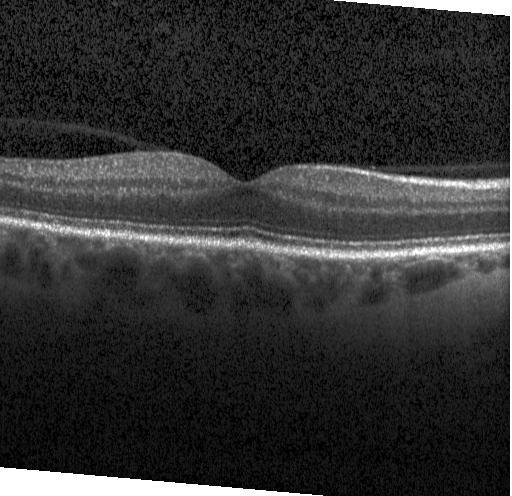
Spectral-domain optical coherence tomography; OCT line scan; through the macula; Heidelberg Spectralis OCT system — Macular OCT: no evidence of CNV, DME, or drusen.